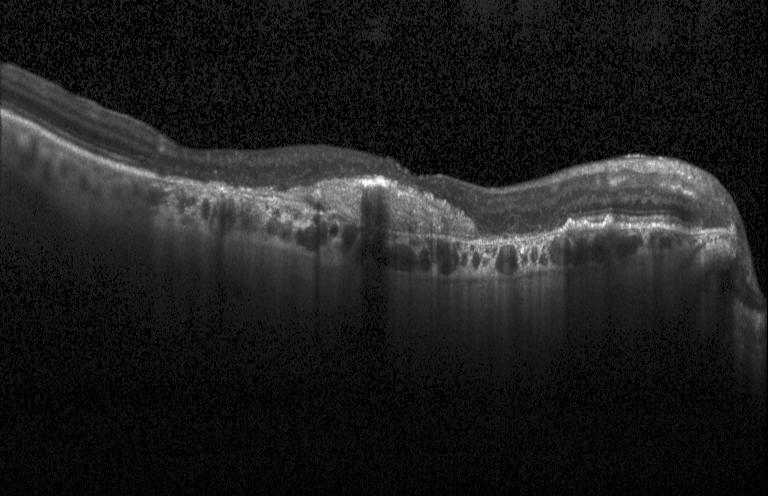 The scan shows choroidal neovascularization.